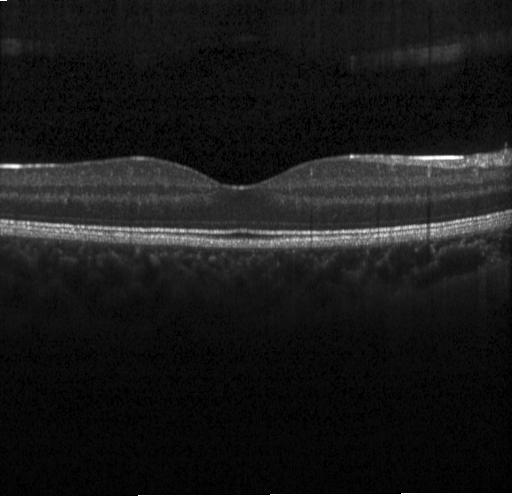
Macular OCT demonstrating no CNV, DME, or drusen.